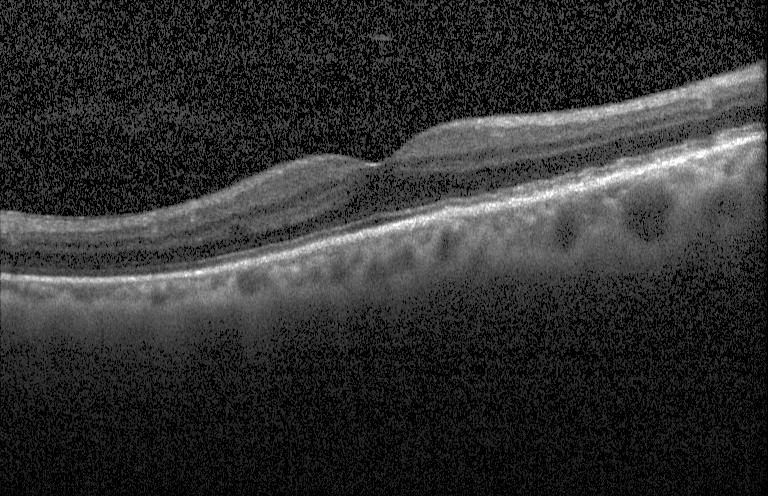

The scan shows no choroidal neovascularization, diabetic macular edema, or drusen.